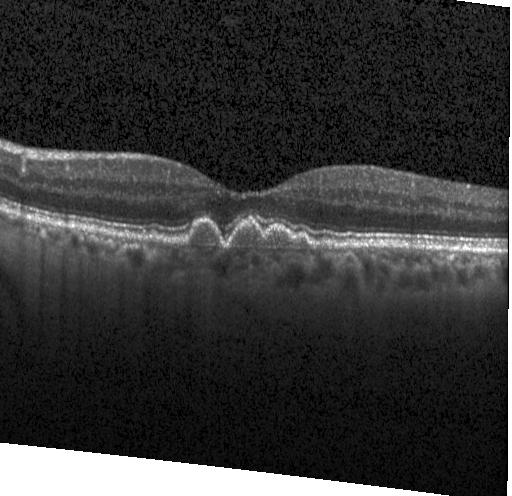
OCT B-scan. Macular scan. Spectral-domain OCT.
Assessment: sub-RPE drusenoid deposits.